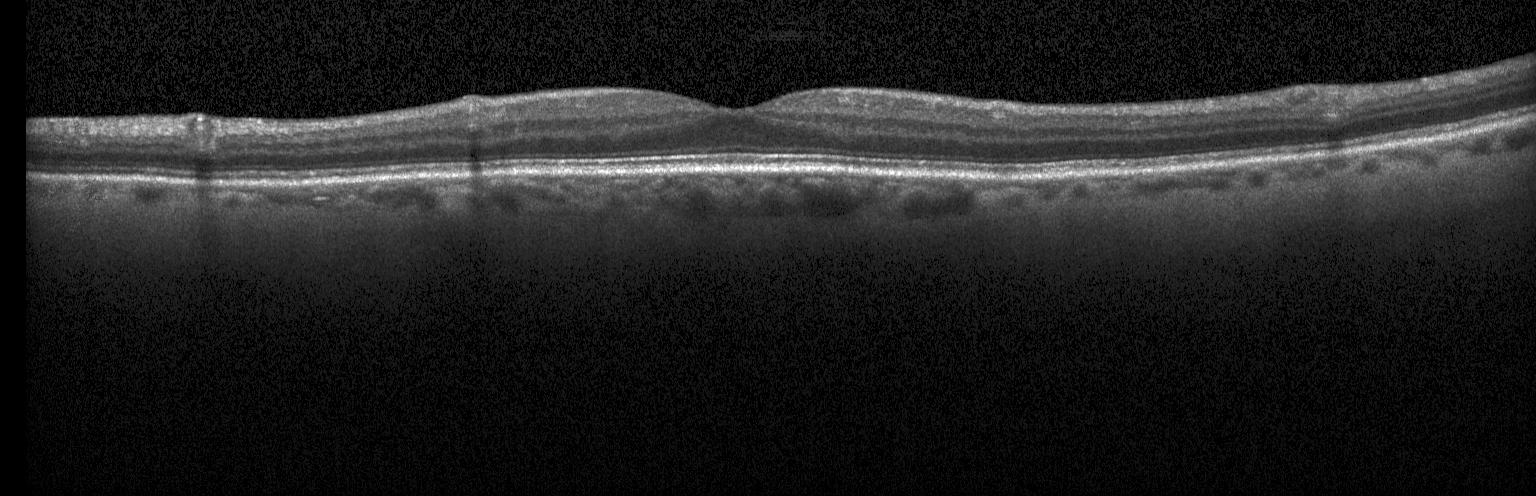

OCT finding: neither CNV, DME, nor drusen.